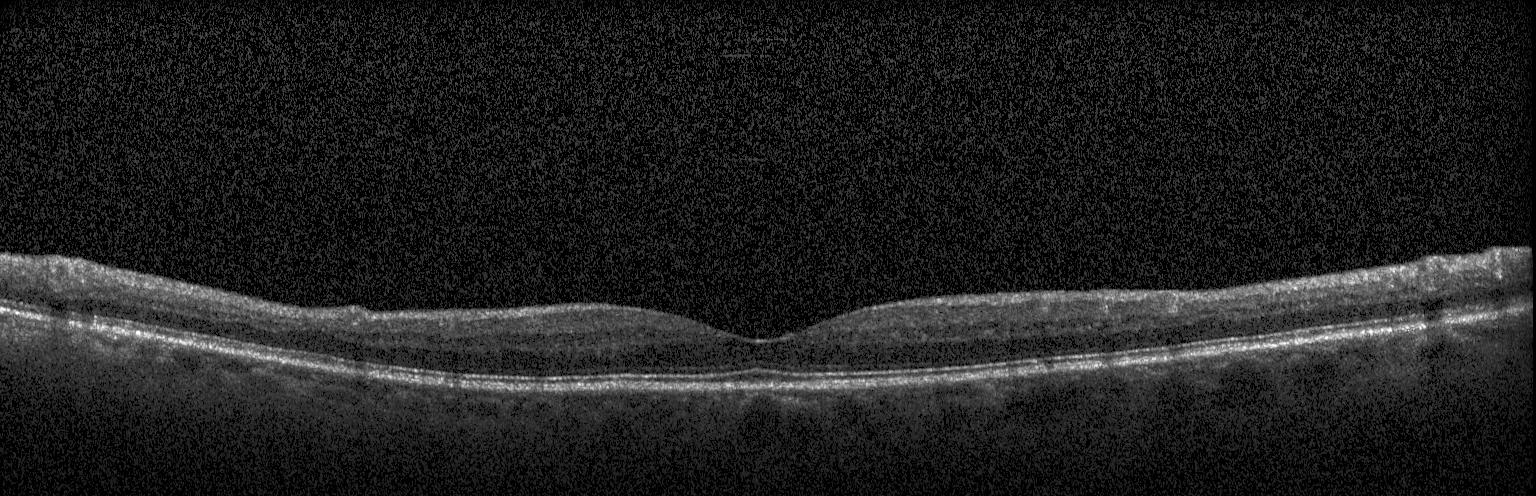
Dx: no CNV, DME, or drusen.